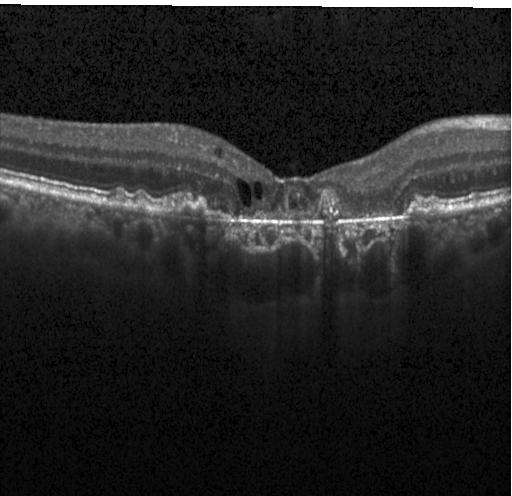 Optical coherence tomography B-scan.
Finding: a choroidal neovascular membrane.